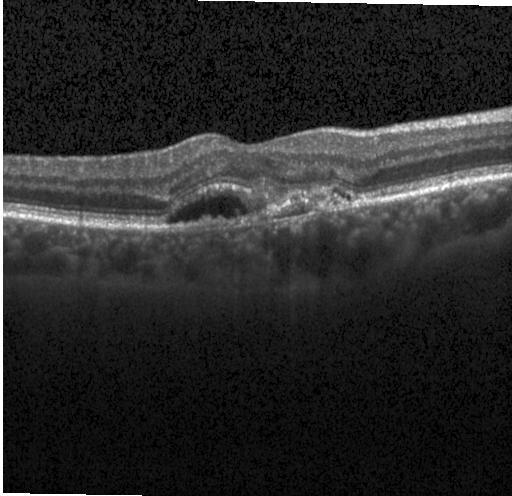
OCT line scan.
Finding: choroidal neovascularization (CNV).